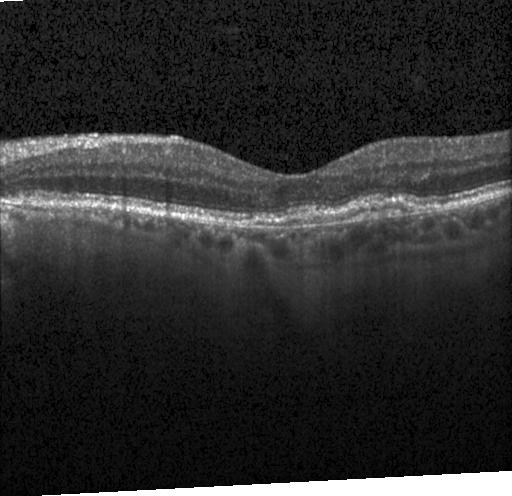

Fovea-centered; OCT line scan; spectral-domain OCT
Impression: choroidal neovascularization.